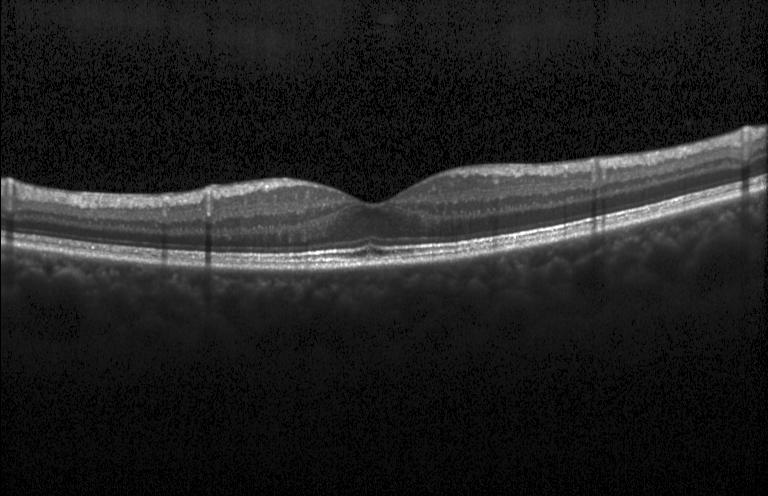

Spectral-domain OCT B-scan: no choroidal neovascularization, diabetic macular edema, or drusen.